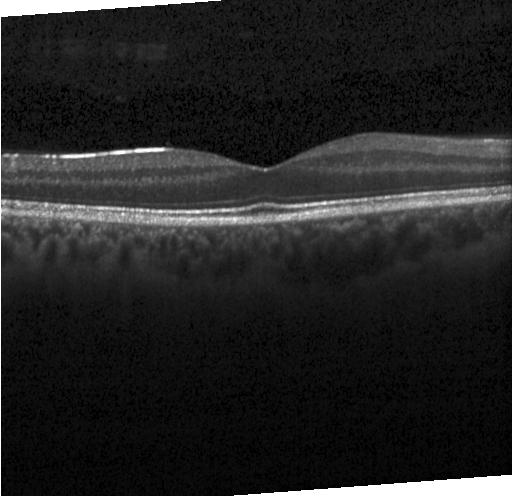
Diagnosis: no CNV, no DME, and no drusen.